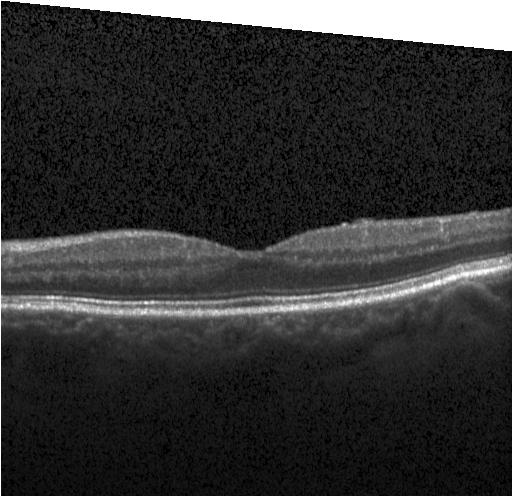

Heidelberg Spectralis OCT system; SD-OCT; OCT B-scan; macular scan
Impression: no choroidal neovascularization, no diabetic macular edema, and no drusen.